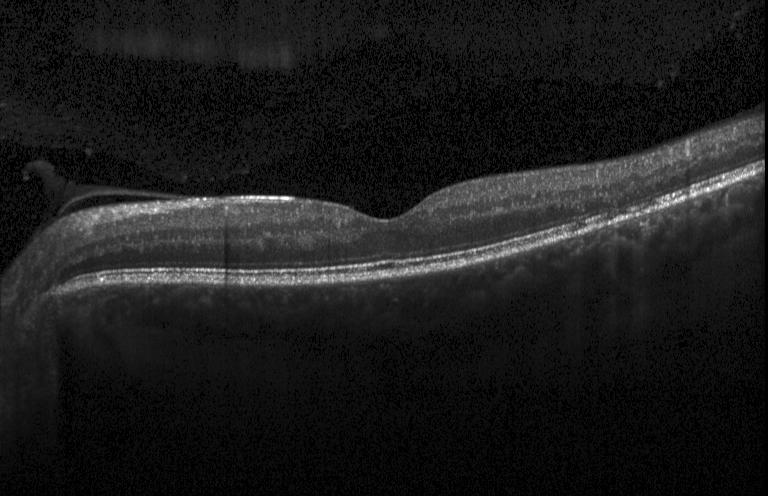
Fovea-centered. OCT B-scan
This B-scan demonstrates no choroidal neovascularization, no diabetic macular edema, and no drusen.